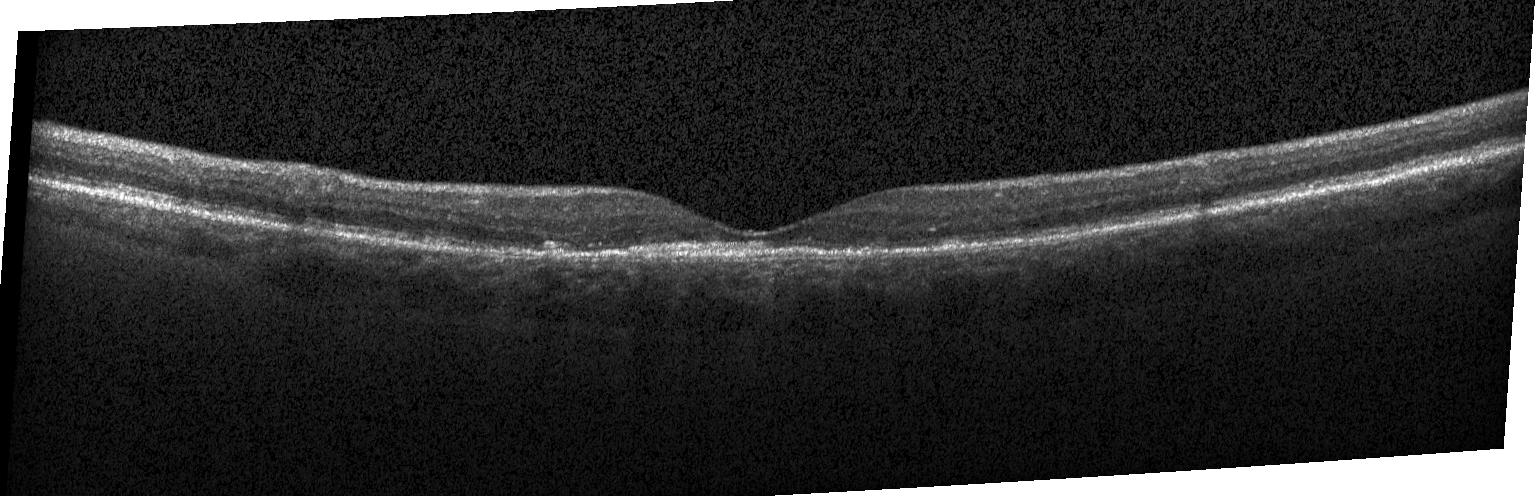 Diagnosis: a choroidal neovascular membrane.